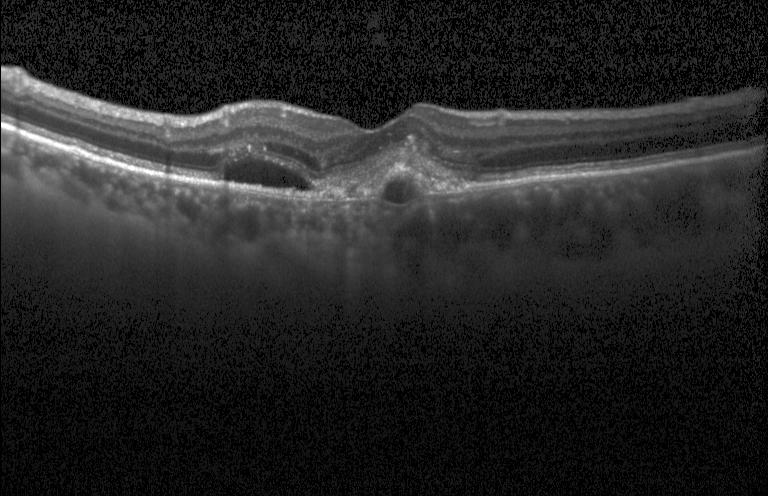 OCT finding: CNV.